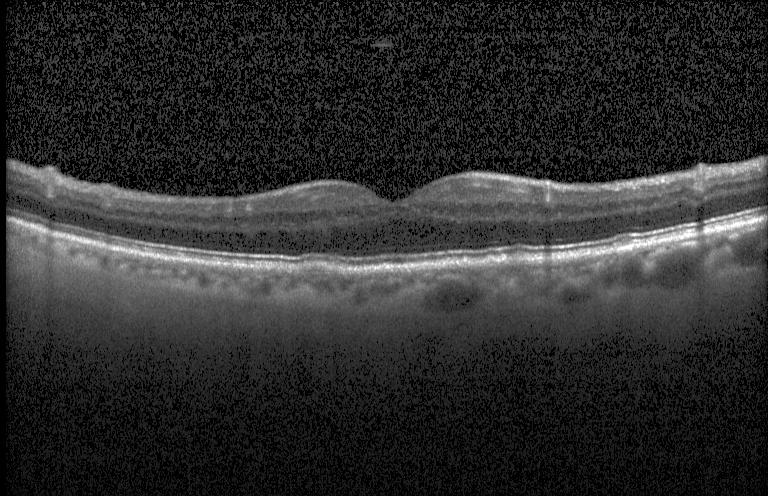 Spectral-domain OCT B-scan: sub-RPE drusenoid deposits.